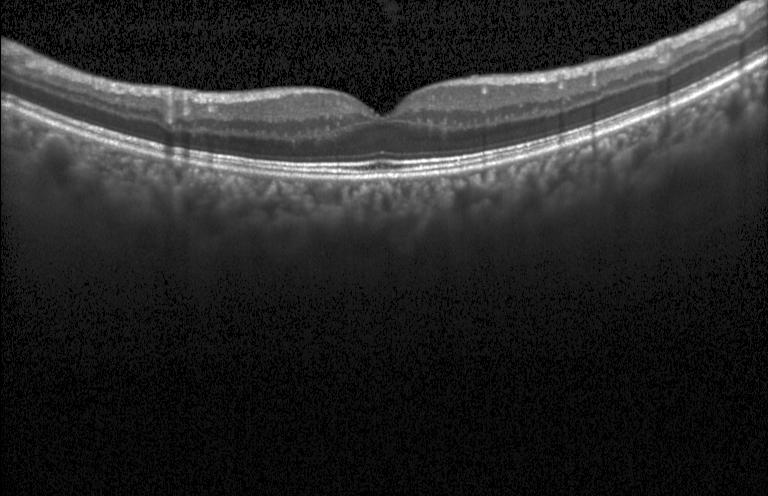
OCT line scan; centered on the fovea; spectral-domain OCT; Heidelberg Spectralis OCT system.
Assessment: no evidence of CNV, DME, or drusen.